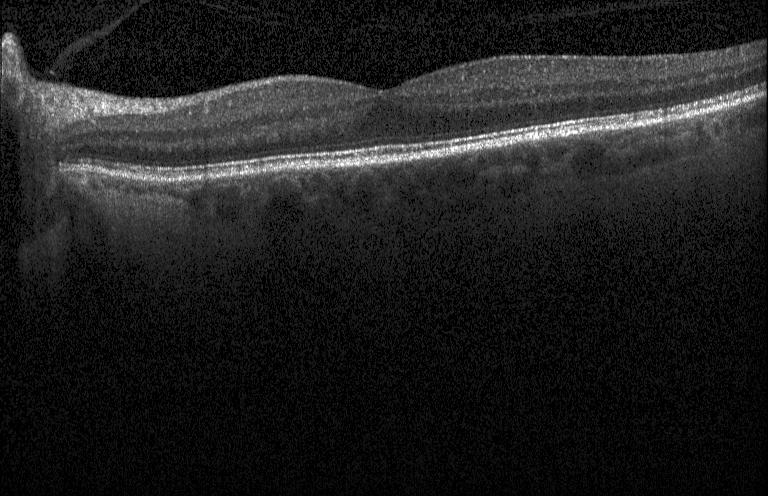 Finding: no evidence of choroidal neovascularization, diabetic macular edema, or drusen.